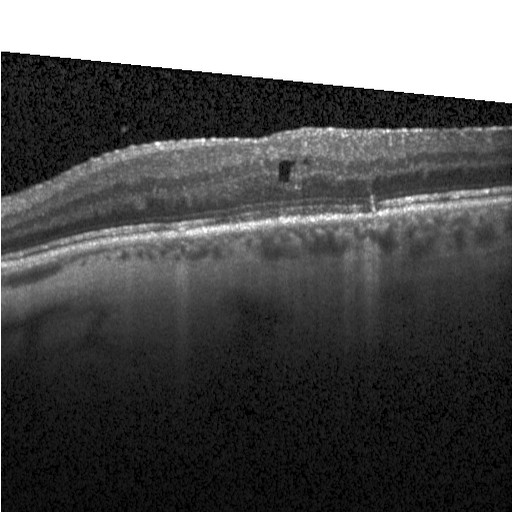

OCT line scan. Spectral-domain OCT. Through the macula
Dx: DME.